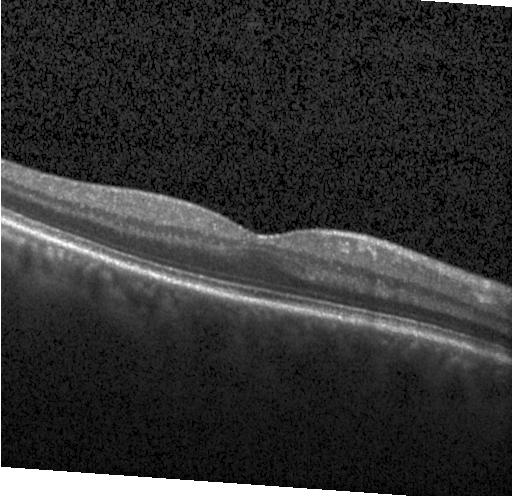
Centered on the fovea · acquired on a Heidelberg Spectralis · optical coherence tomography scan — This B-scan demonstrates no choroidal neovascularization, no diabetic macular edema, and no drusen.